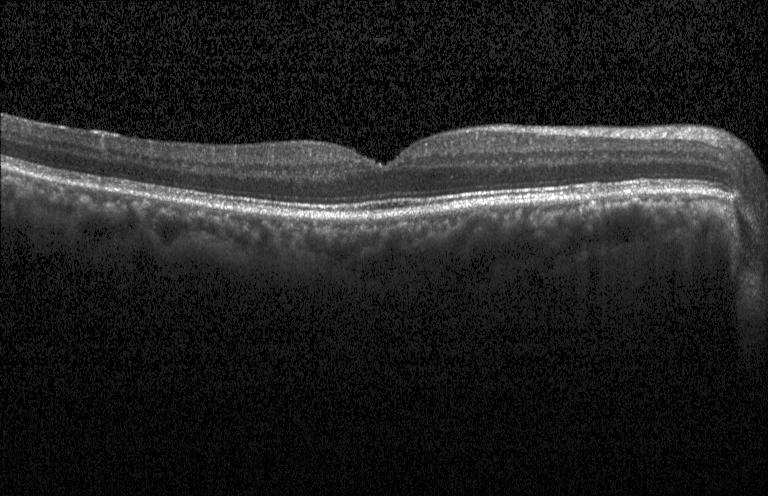 Spectral-domain optical coherence tomography. Horizontal scan through the fovea. OCT line scan — Impression: no choroidal neovascularization, no diabetic macular edema, and no drusen.